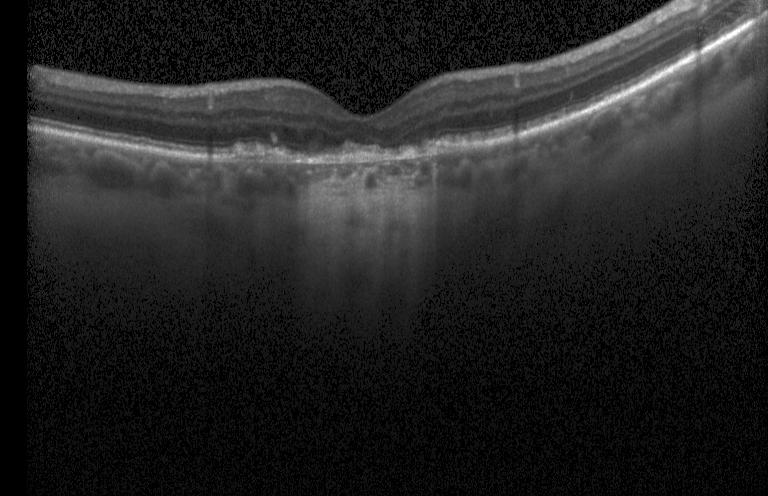

Diagnosis: a choroidal neovascular membrane.